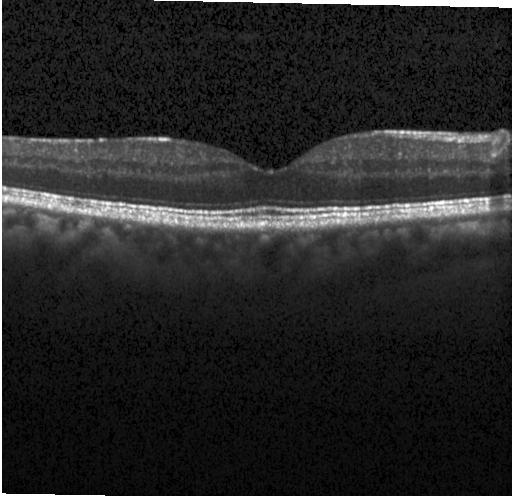 Centered on the fovea. OCT B-scan.
Impression: neither CNV, DME, nor drusen.